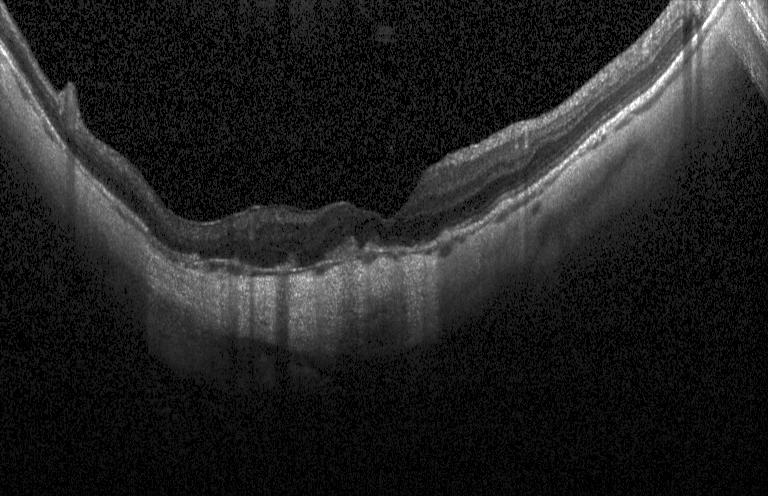
Spectral-domain optical coherence tomography; horizontal scan through the fovea; retinal OCT B-scan. Impression: a choroidal neovascular membrane.